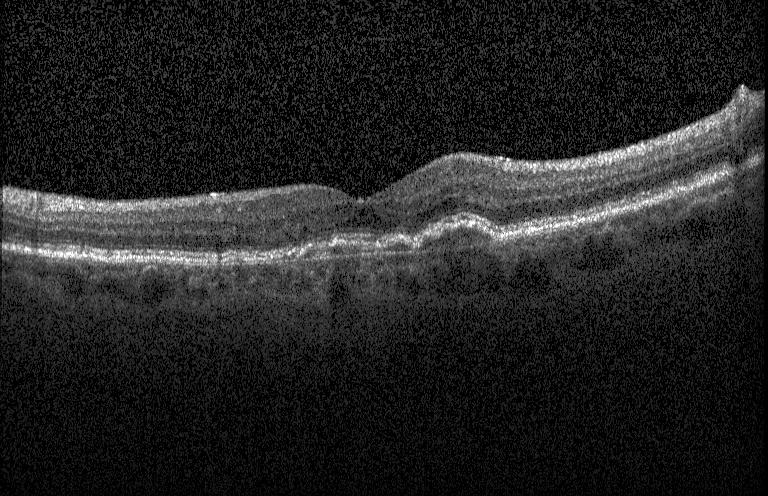 Diagnosis: choroidal neovascularization.